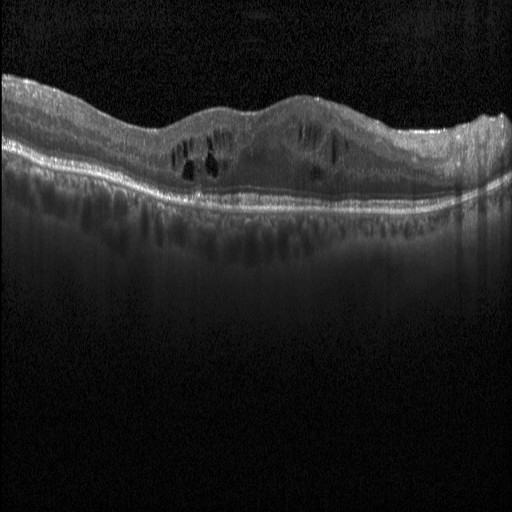

OCT line scan — Impression: DME.